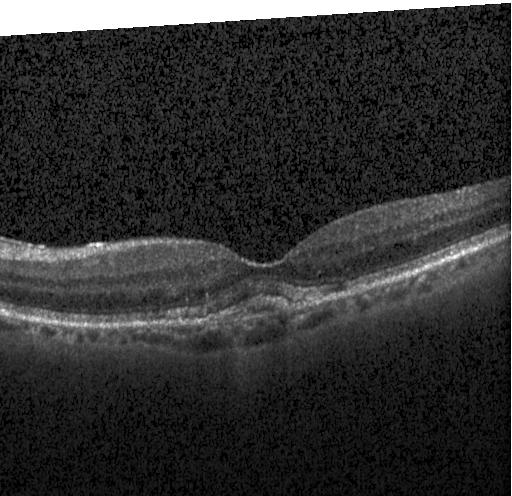 SD-OCT · retinal OCT B-scan — This B-scan demonstrates a choroidal neovascular membrane.